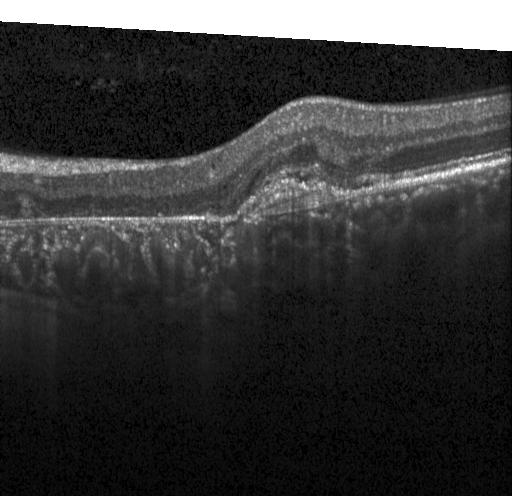

OCT B-scan, spectral-domain optical coherence tomography, centered on the fovea, instrument: Heidelberg Spectralis.
Assessment: CNV.